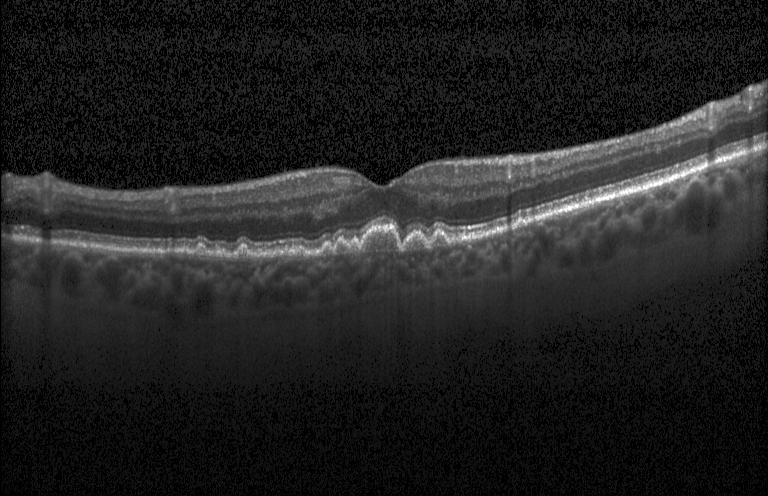 Optical coherence tomography scan, spectral-domain optical coherence tomography — Sub-RPE drusenoid deposits.